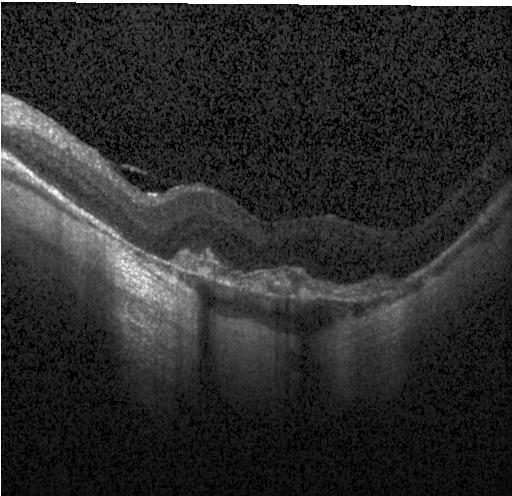

Impression: a choroidal neovascular membrane.